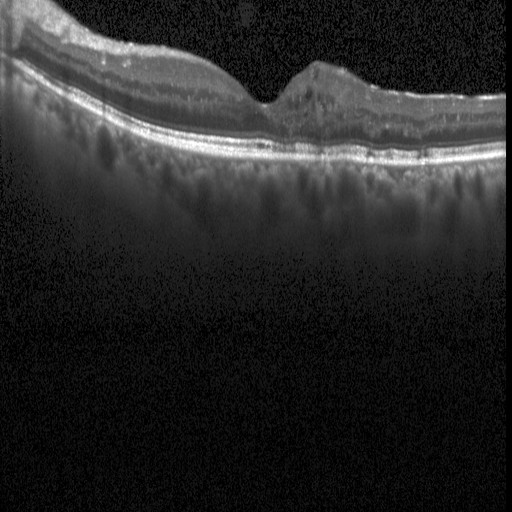

Impression: DME.